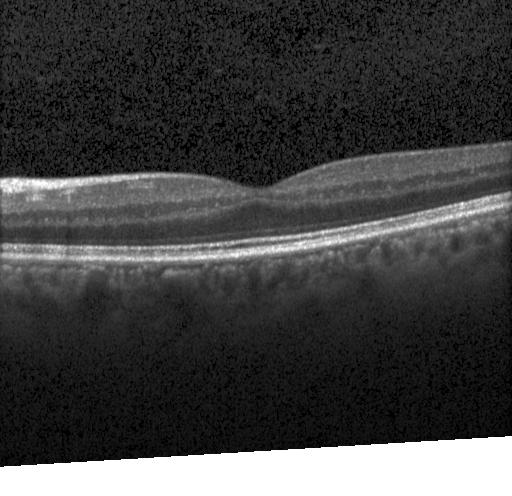
SD-OCT. Optical coherence tomography scan. Instrument: Heidelberg Spectralis. Through the macula.
This B-scan demonstrates no choroidal neovascularization, diabetic macular edema, or drusen.